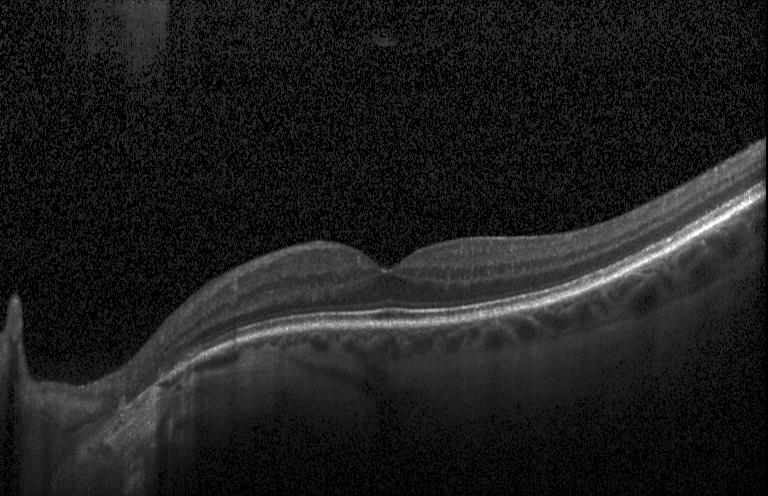
Optical coherence tomography B-scan.
Finding: neither CNV, DME, nor drusen.